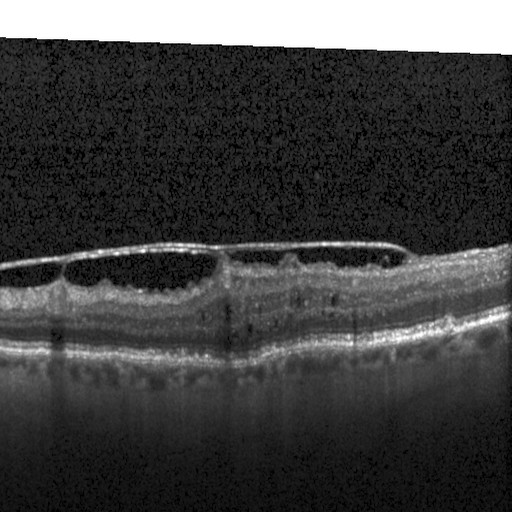

Retinal OCT B-scan. Macular scan. Spectral-domain optical coherence tomography. Instrument: Heidelberg Spectralis. OCT finding: diabetic macular edema (DME).